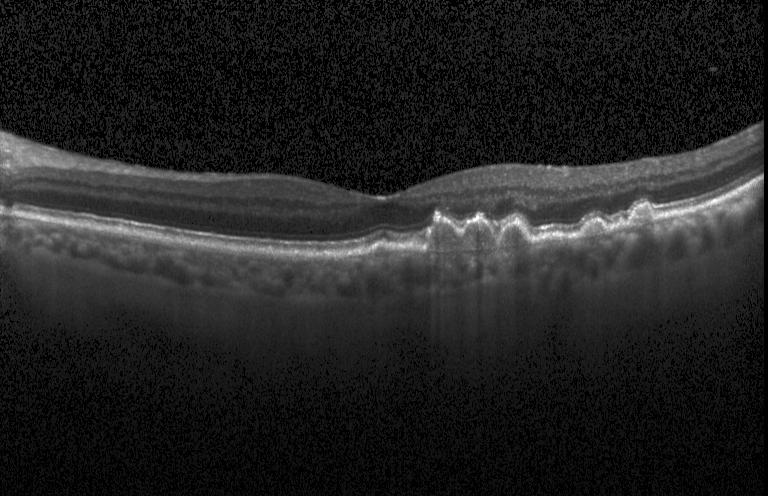 Impression: sub-RPE drusenoid deposits.